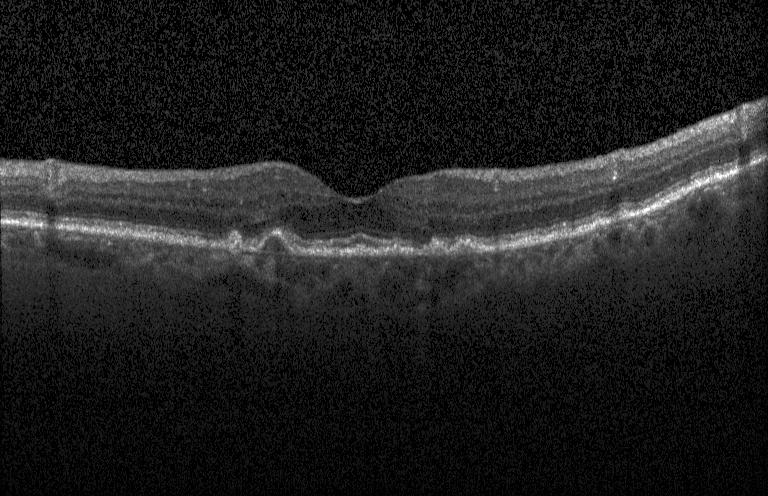 Retinal OCT B-scan · SD-OCT · macular scan — Finding: drusen.